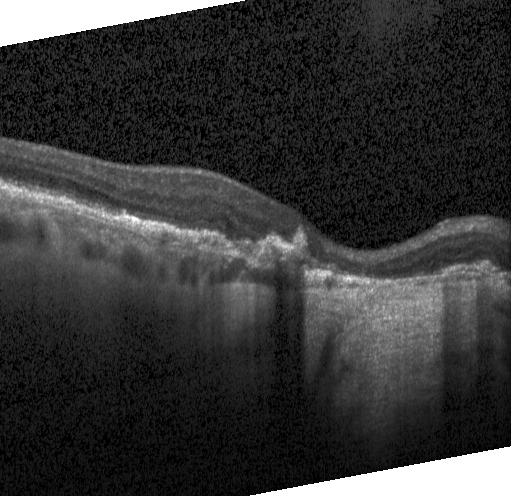
Centered on the fovea, OCT B-scan
This B-scan demonstrates choroidal neovascularization.